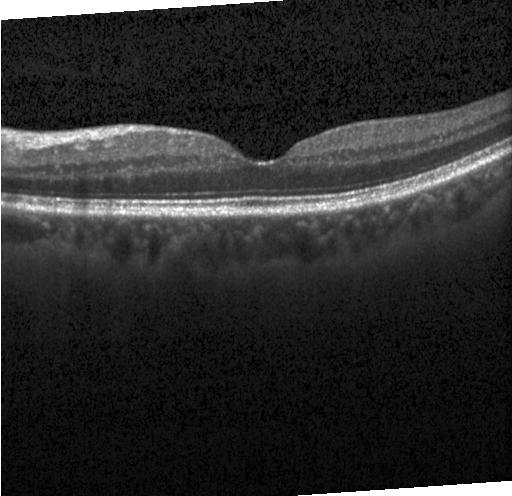
Diagnosis: no choroidal neovascularization, no diabetic macular edema, and no drusen.